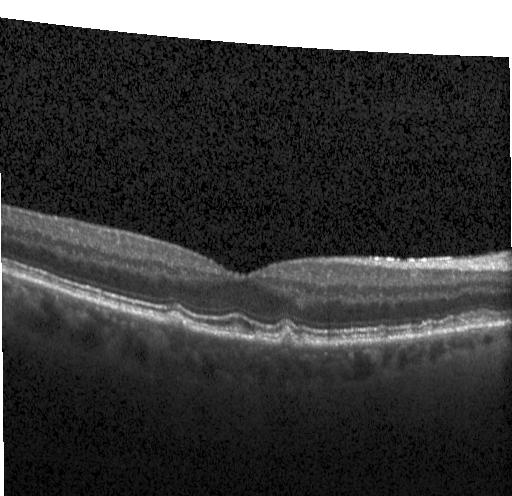
OCT line scan.
Assessment: sub-RPE drusenoid deposits.